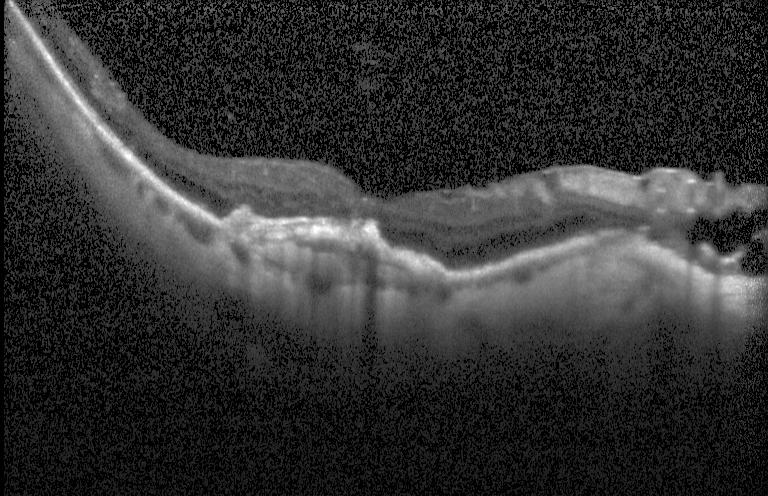
Optical coherence tomography scan — OCT finding: a choroidal neovascular membrane.